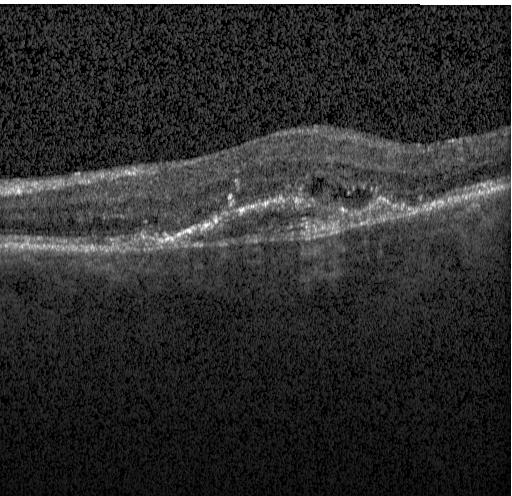
Spectral-domain optical coherence tomography. OCT line scan. Heidelberg Spectralis OCT system.
Diagnosis: a choroidal neovascular membrane.